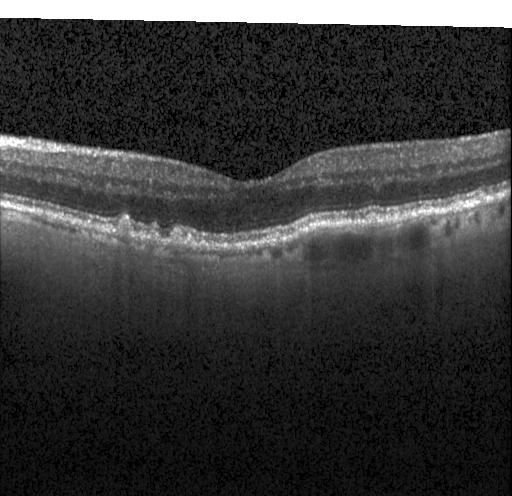 Heidelberg Spectralis · optical coherence tomography scan · SD-OCT.
This B-scan demonstrates drusen.